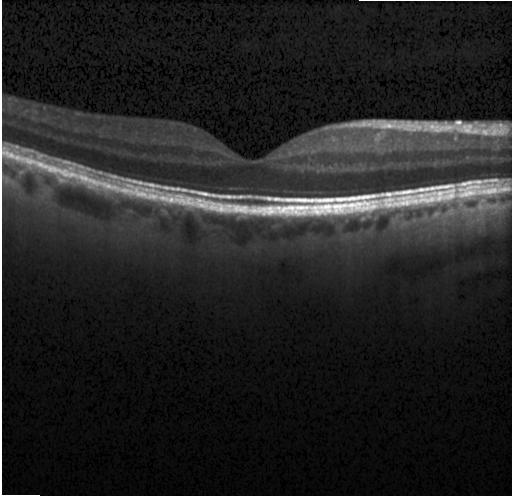
Diagnosis: no evidence of choroidal neovascularization, diabetic macular edema, or drusen.